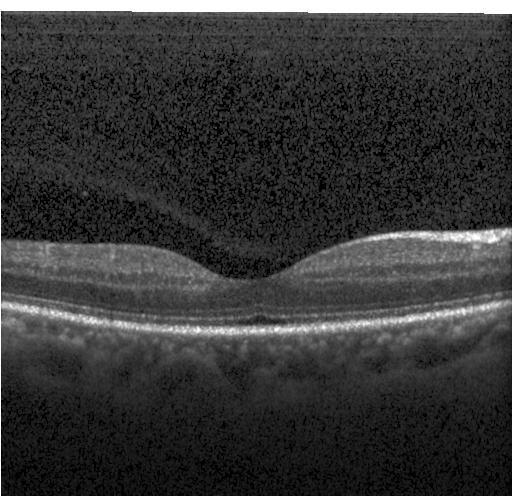 OCT B-scan
Diagnosis: no choroidal neovascularization, no diabetic macular edema, and no drusen.